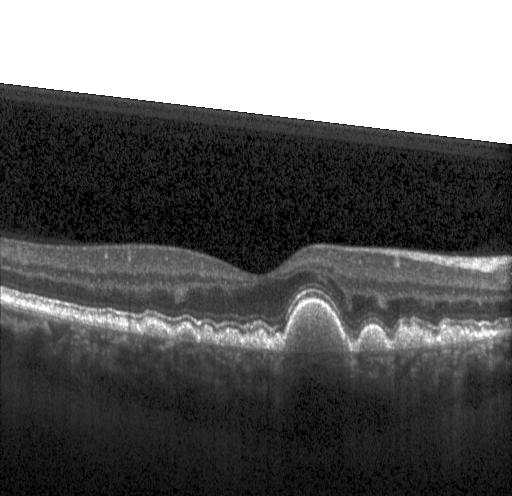
Fovea-centered · OCT B-scan · Heidelberg Spectralis OCT system — Finding: sub-RPE drusenoid deposits.